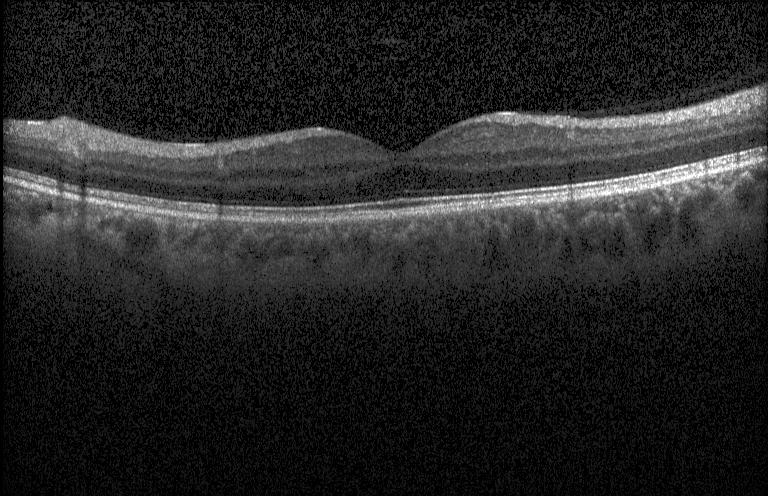

No evidence of choroidal neovascularization, diabetic macular edema, or drusen.